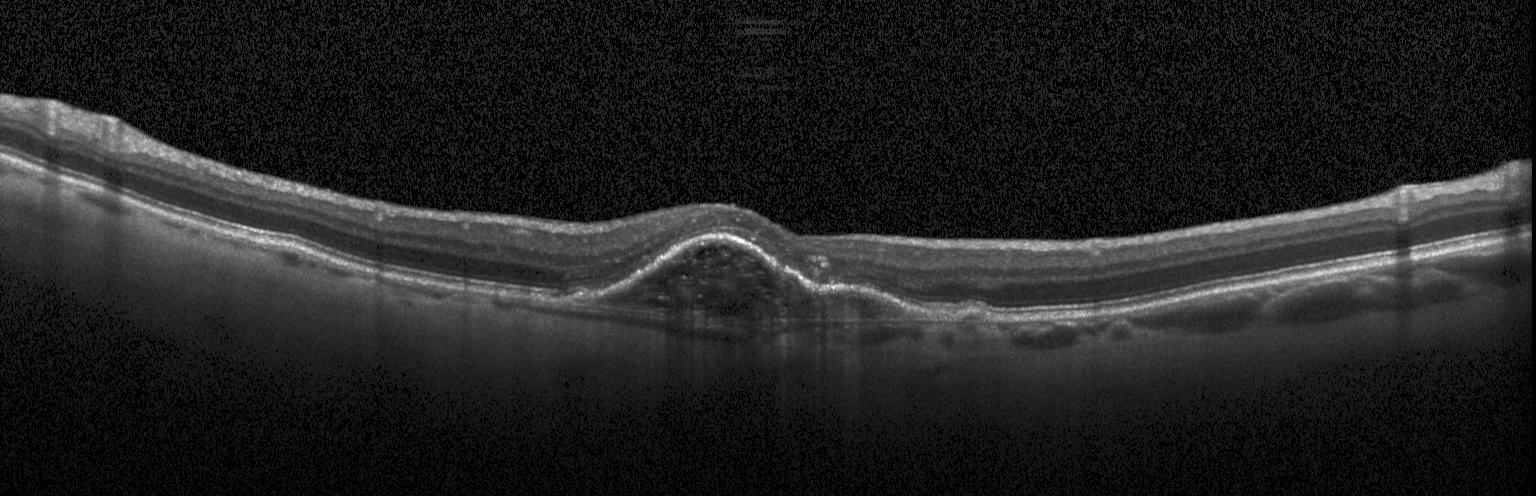 Horizontal scan through the fovea; retinal OCT cross-section. The scan shows choroidal neovascularization (CNV).